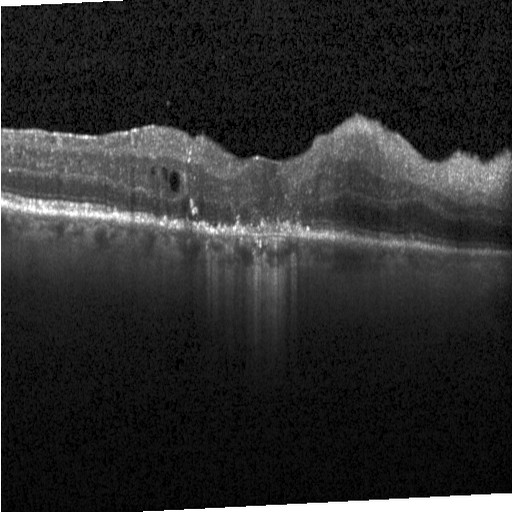
Diagnosis: diabetic macular edema (DME).